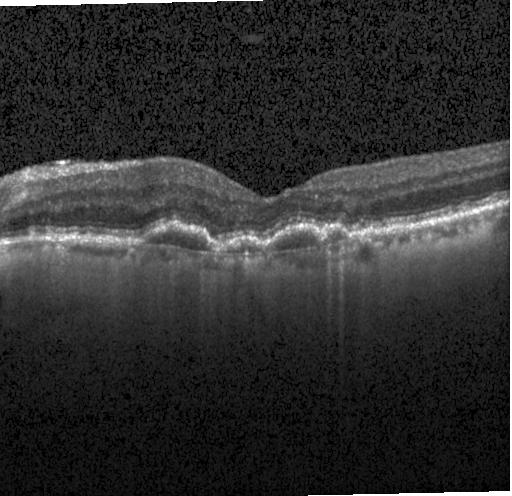
A choroidal neovascular membrane.